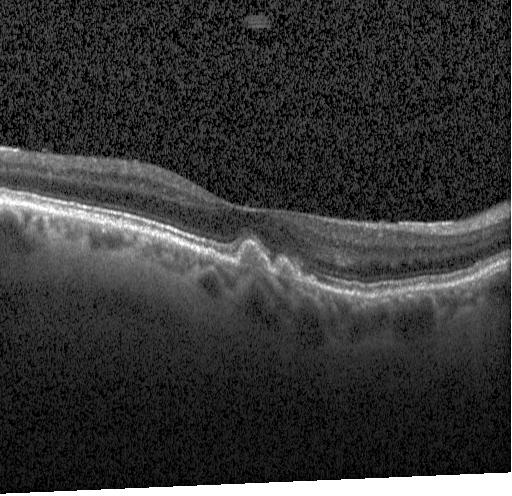 Diagnosis: sub-RPE drusenoid deposits.